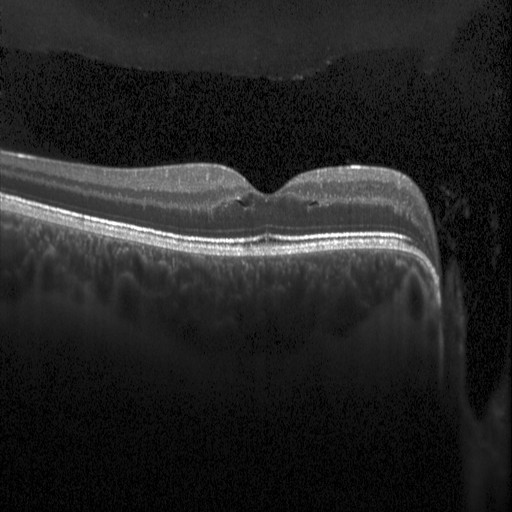

Fovea-centered · optical coherence tomography B-scan · spectral-domain OCT · instrument: Heidelberg Spectralis — Diagnosis: DME.